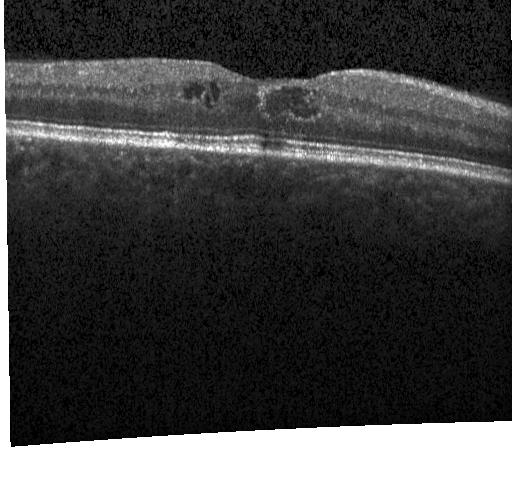 Diagnosis: diabetic macular edema (DME).